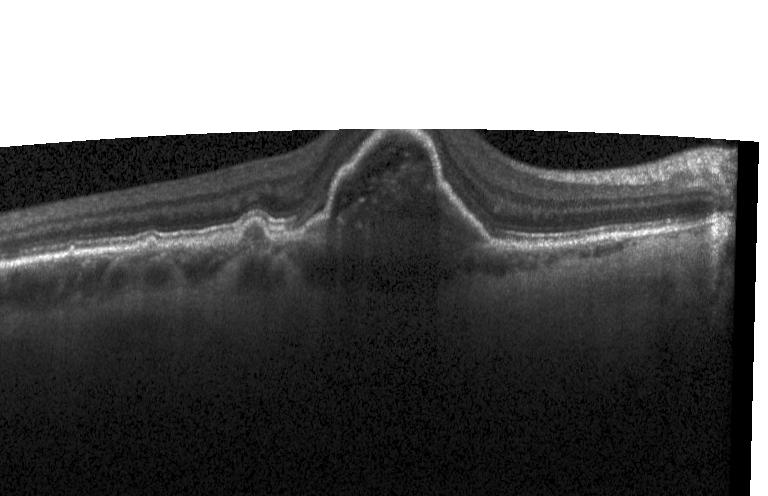

Retinal OCT cross-section showing a choroidal neovascular membrane.